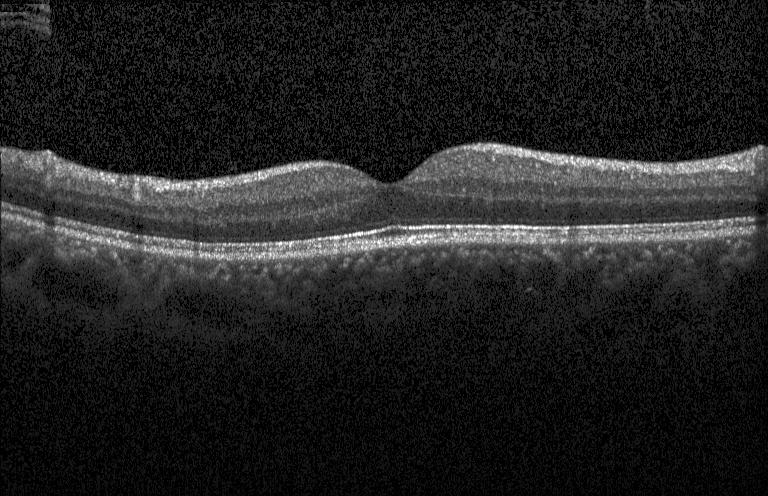
Spectral-domain optical coherence tomography, Heidelberg Spectralis, retinal OCT cross-section. Impression: no evidence of choroidal neovascularization, diabetic macular edema, or drusen.